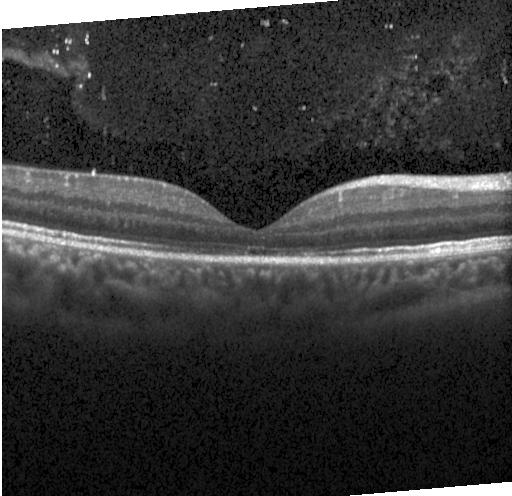
Through the macula · OCT B-scan · instrument: Heidelberg Spectralis. Impression: no choroidal neovascularization, diabetic macular edema, or drusen.